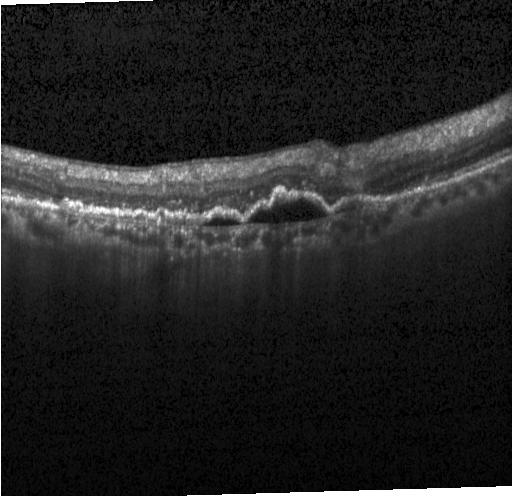 SD-OCT · OCT line scan
Macular OCT: a choroidal neovascular membrane.